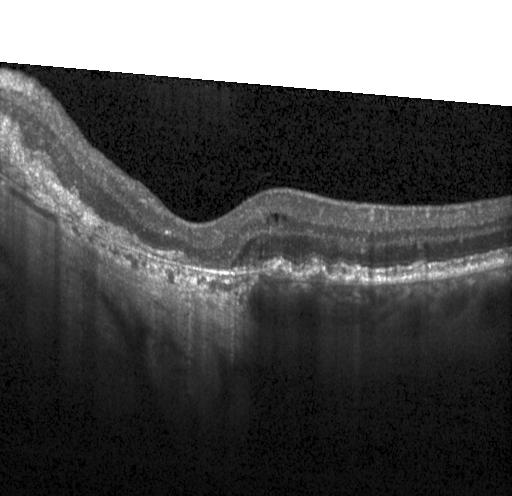

Retinal OCT cross-section — Dx: a choroidal neovascular membrane.